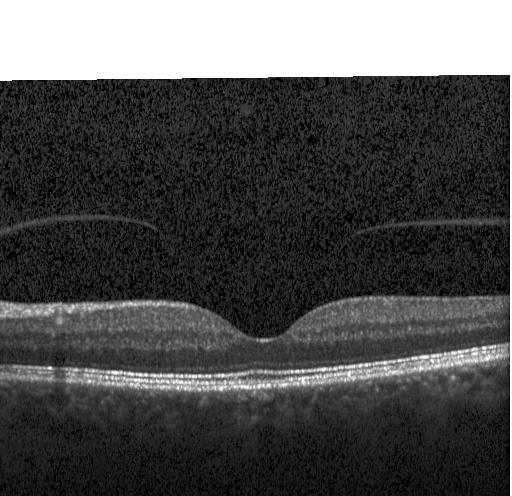
Retinal OCT cross-section, fovea-centered, SD-OCT — No evidence of choroidal neovascularization, diabetic macular edema, or drusen.